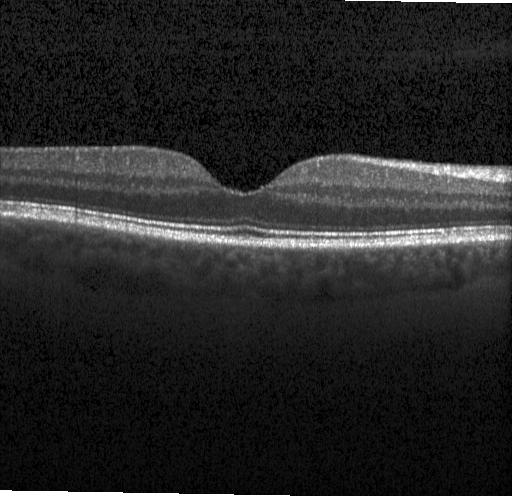
Heidelberg Spectralis OCT system; optical coherence tomography B-scan; spectral-domain OCT — Diagnosis: no choroidal neovascularization, no diabetic macular edema, and no drusen.